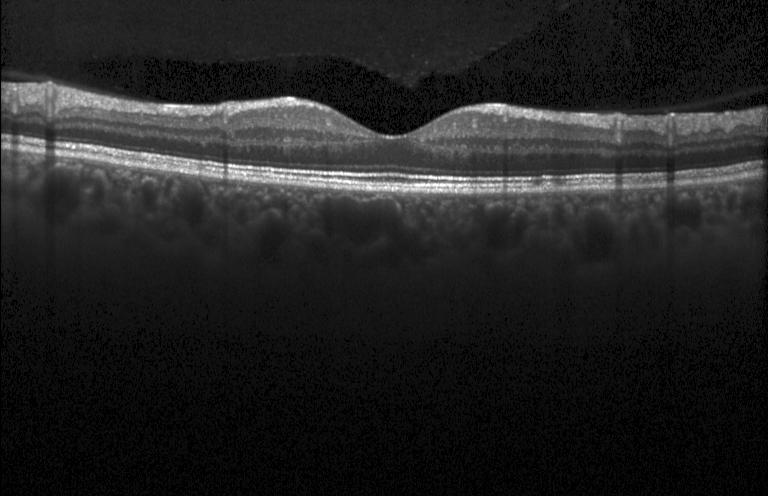
Dx: neither choroidal neovascularization, diabetic macular edema, nor drusen.